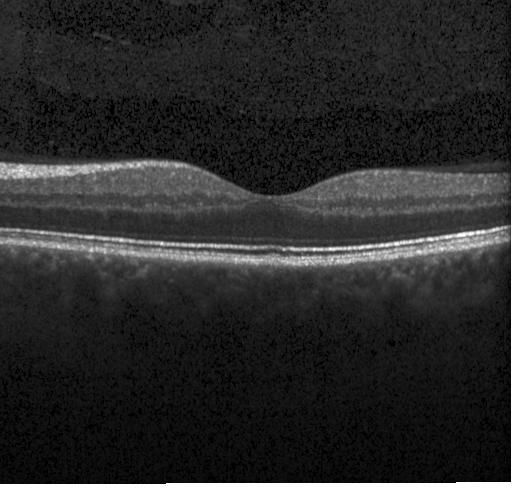 Optical coherence tomography B-scan
Impression: no choroidal neovascularization, diabetic macular edema, or drusen.